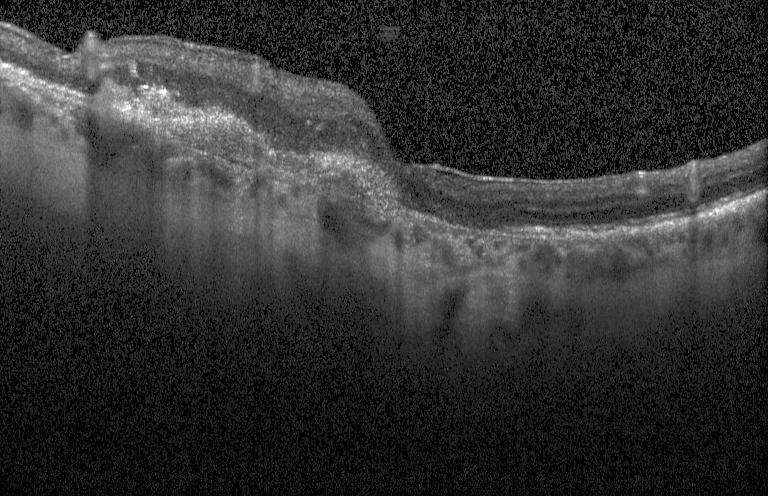 Dx: a choroidal neovascular membrane.